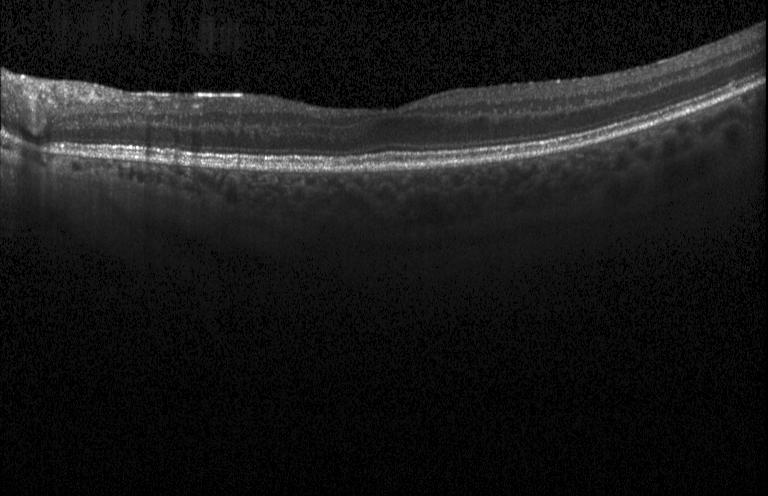

Heidelberg Spectralis. Horizontal scan through the fovea. SD-OCT. Optical coherence tomography scan.
Finding: neither CNV, DME, nor drusen.